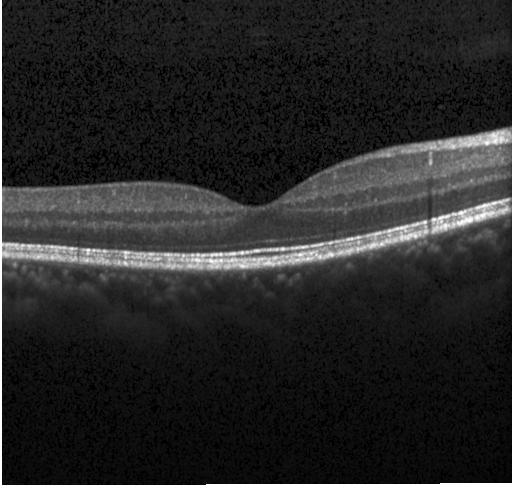 Macular OCT: no choroidal neovascularization, diabetic macular edema, or drusen.